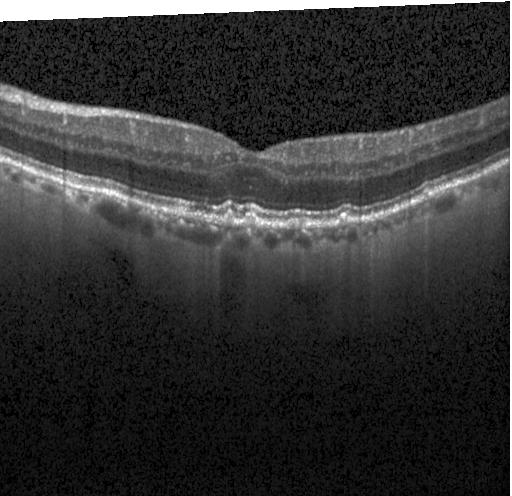 Retinal OCT cross-section · Heidelberg Spectralis · spectral-domain optical coherence tomography. Sub-RPE drusenoid deposits.